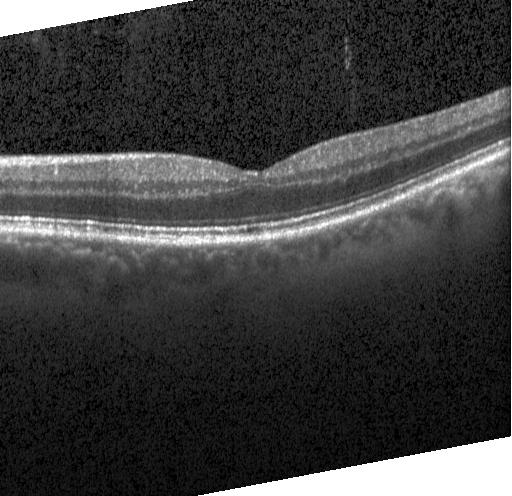 Retinal OCT cross-section
Neither choroidal neovascularization, diabetic macular edema, nor drusen.